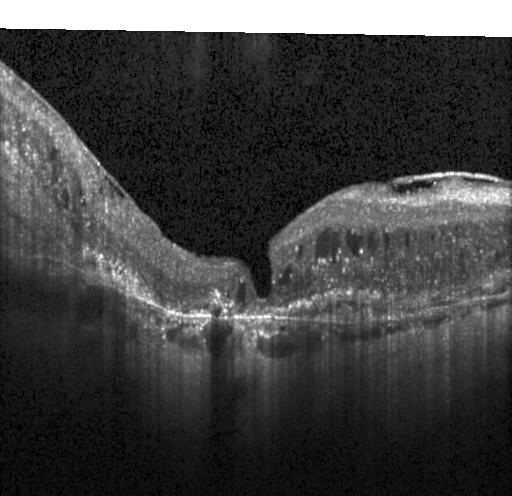

OCT scan showing CNV.